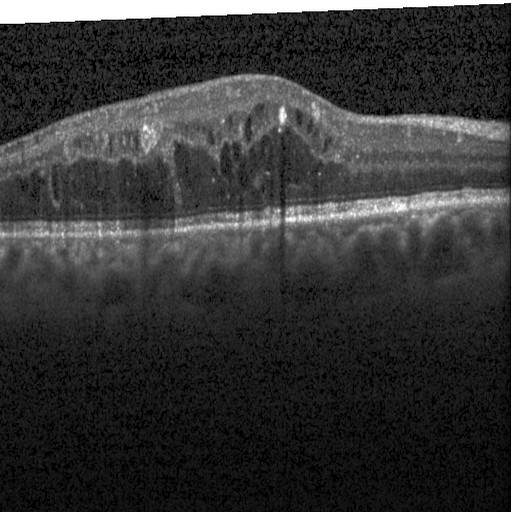

Optical coherence tomography B-scan · fovea-centered.
OCT finding: DME.